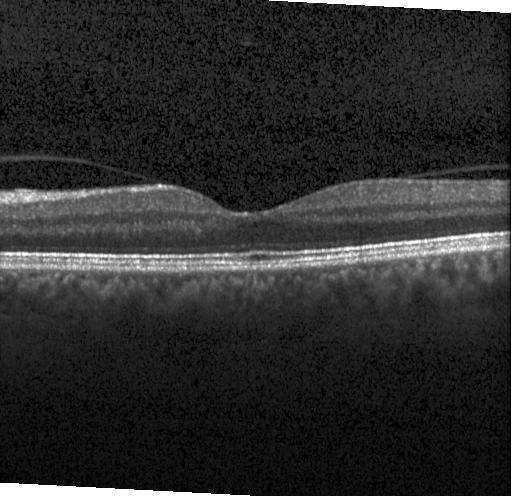

OCT B-scan.
This B-scan demonstrates no choroidal neovascularization, diabetic macular edema, or drusen.